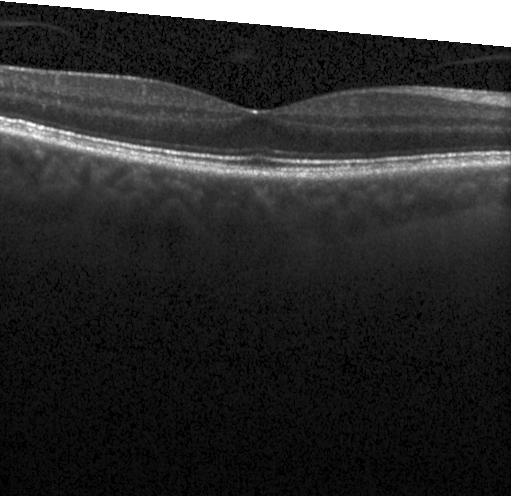
Spectral-domain optical coherence tomography, optical coherence tomography B-scan, macular scan
Finding: no CNV, DME, or drusen.